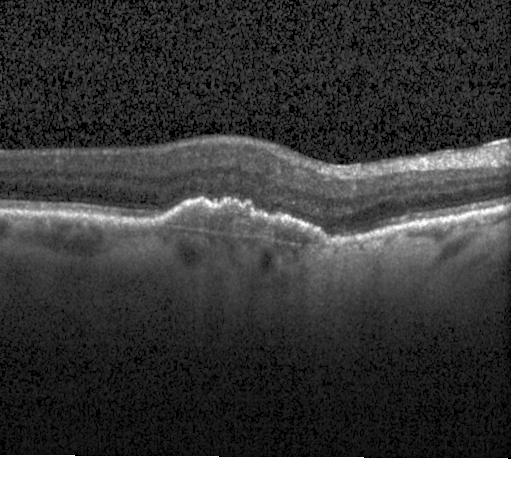

Spectral-domain optical coherence tomography; optical coherence tomography scan; fovea-centered; acquired on a Heidelberg Spectralis. Diagnosis: choroidal neovascularization.